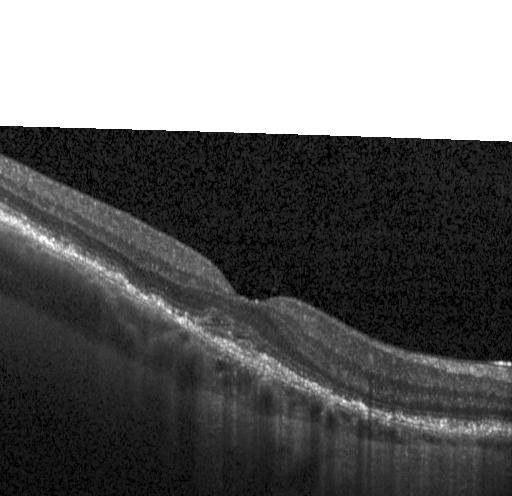
OCT finding: a choroidal neovascular membrane.